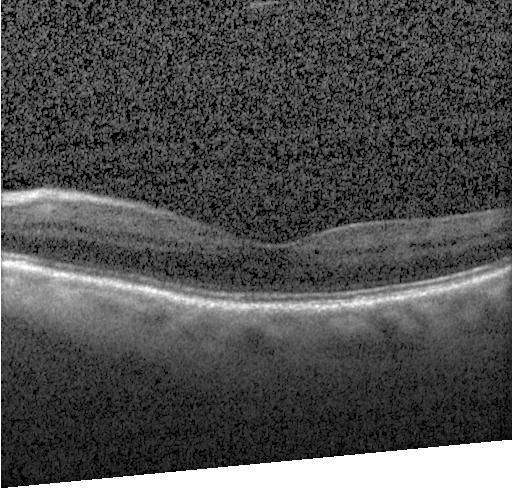

Optical coherence tomography B-scan. Centered on the fovea. Acquired on a Heidelberg Spectralis — Finding: no CNV, DME, or drusen.